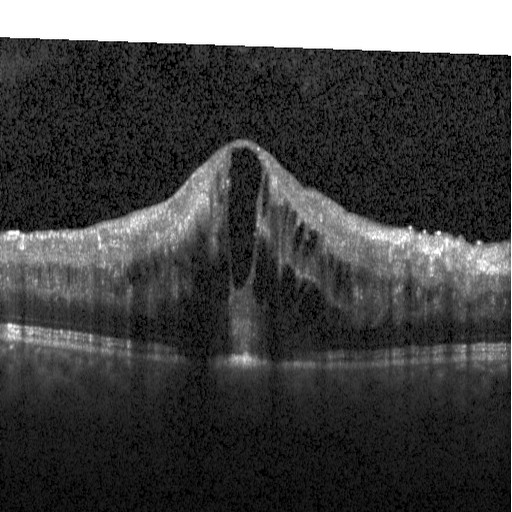

Spectral-domain optical coherence tomography, OCT line scan, through the macula, instrument: Heidelberg Spectralis
This B-scan demonstrates diabetic macular edema (DME).